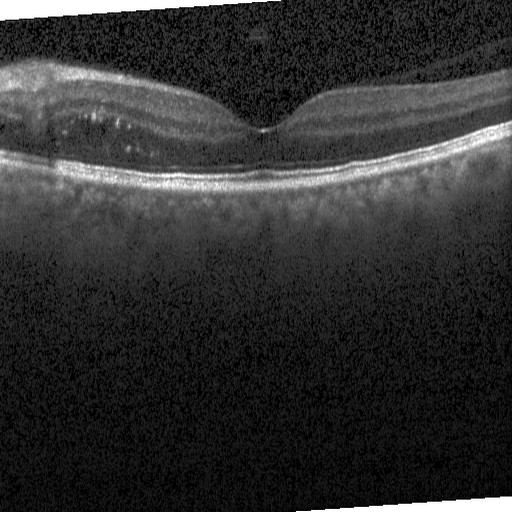
The scan shows diabetic macular edema.